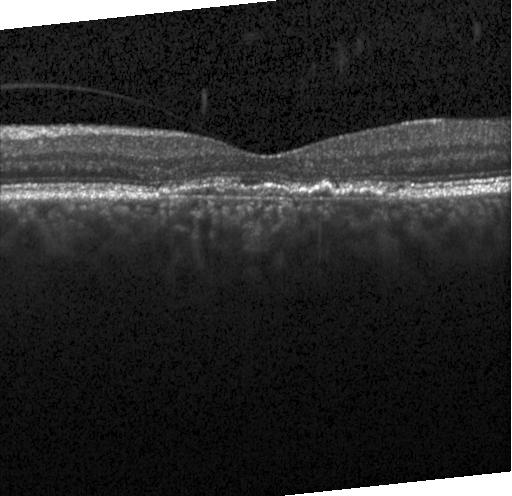

Retinal OCT B-scan, horizontal scan through the fovea. Choroidal neovascularization (CNV).